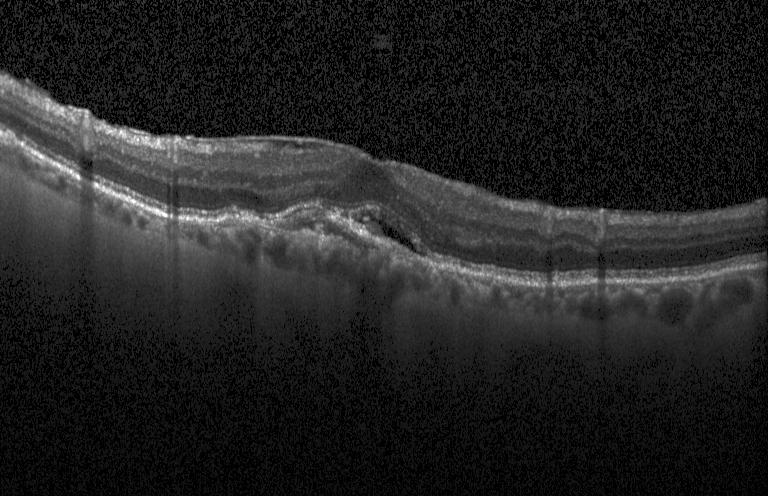
Diagnosis: choroidal neovascularization (CNV).